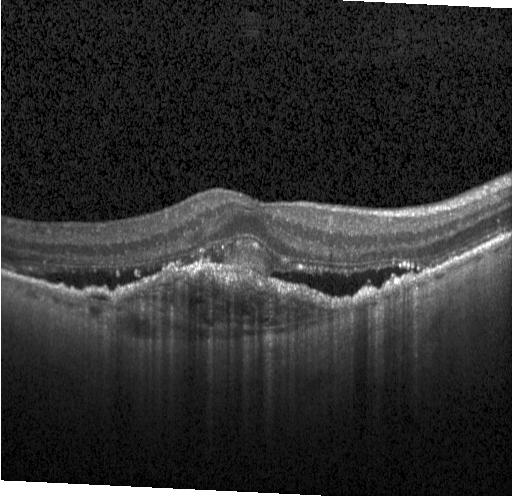
Retinal OCT cross-section showing a choroidal neovascular membrane.